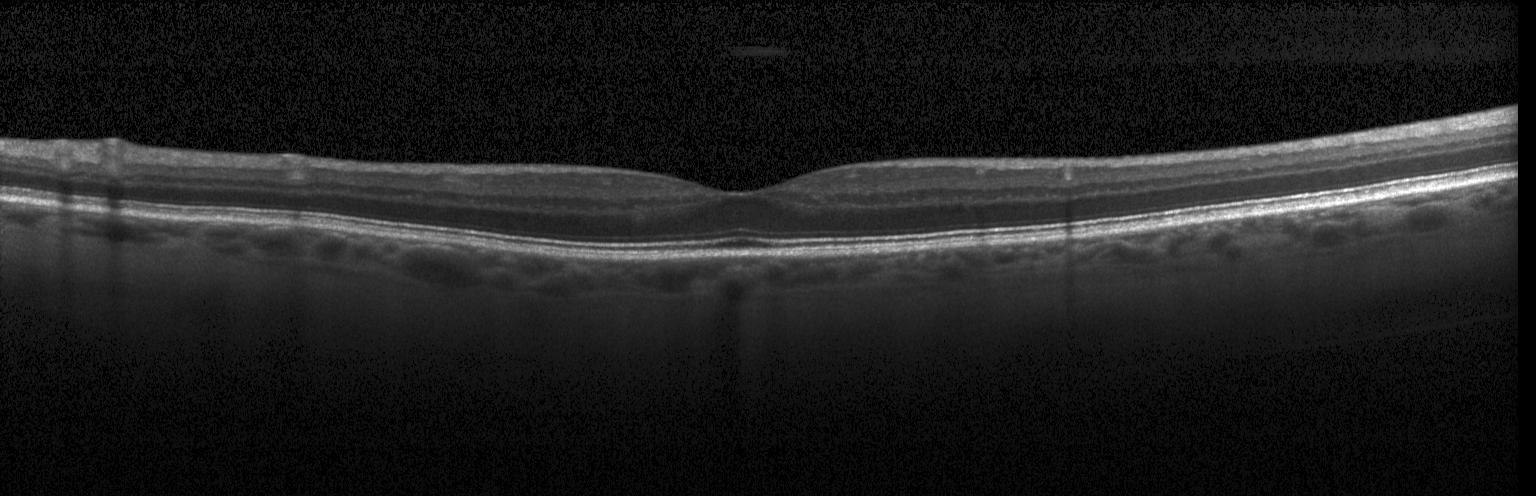 Heidelberg Spectralis OCT system, optical coherence tomography scan, spectral-domain optical coherence tomography, through the macula
Diagnosis: neither choroidal neovascularization, diabetic macular edema, nor drusen.